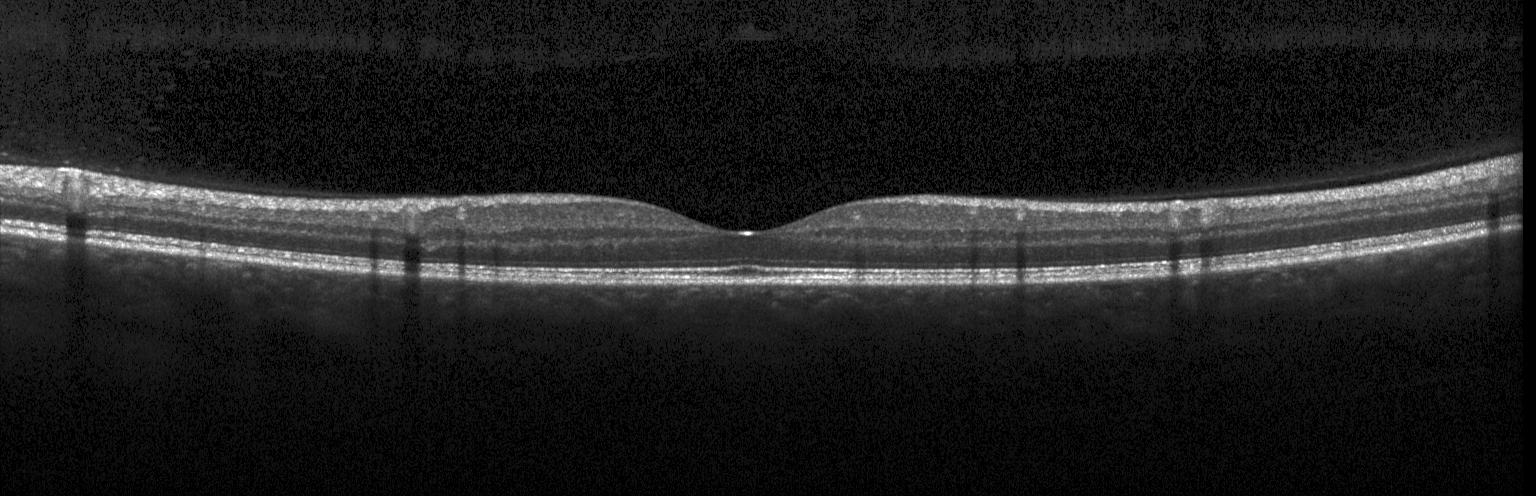
OCT finding: no evidence of choroidal neovascularization, diabetic macular edema, or drusen.